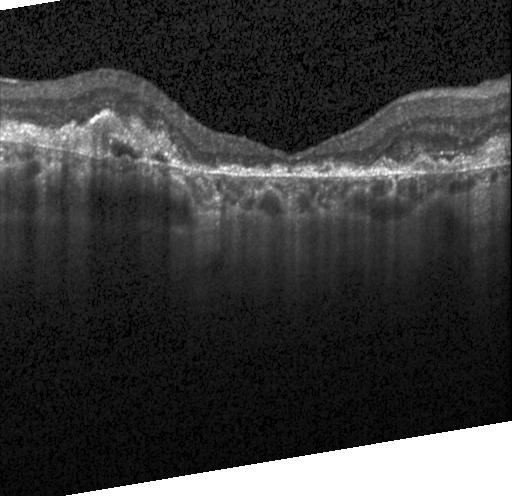 Retinal OCT cross-section. Spectral-domain OCT. Heidelberg Spectralis
Diagnosis: a choroidal neovascular membrane.